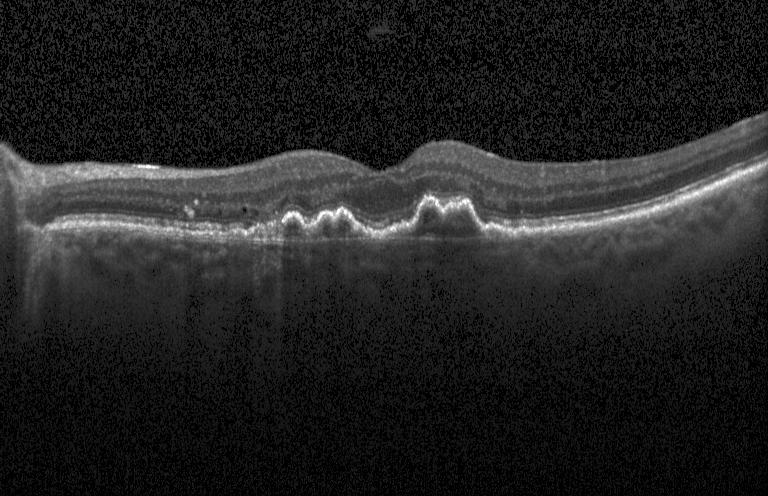 Spectral-domain OCT B-scan: a choroidal neovascular membrane.